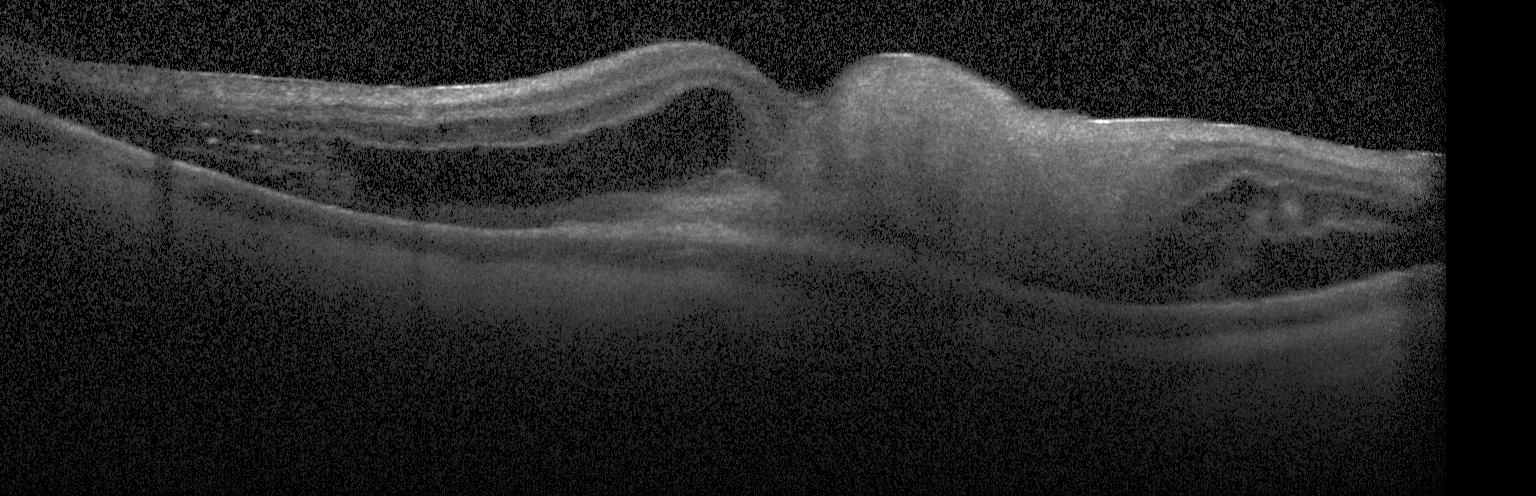

OCT line scan, spectral-domain optical coherence tomography. The scan shows a choroidal neovascular membrane.